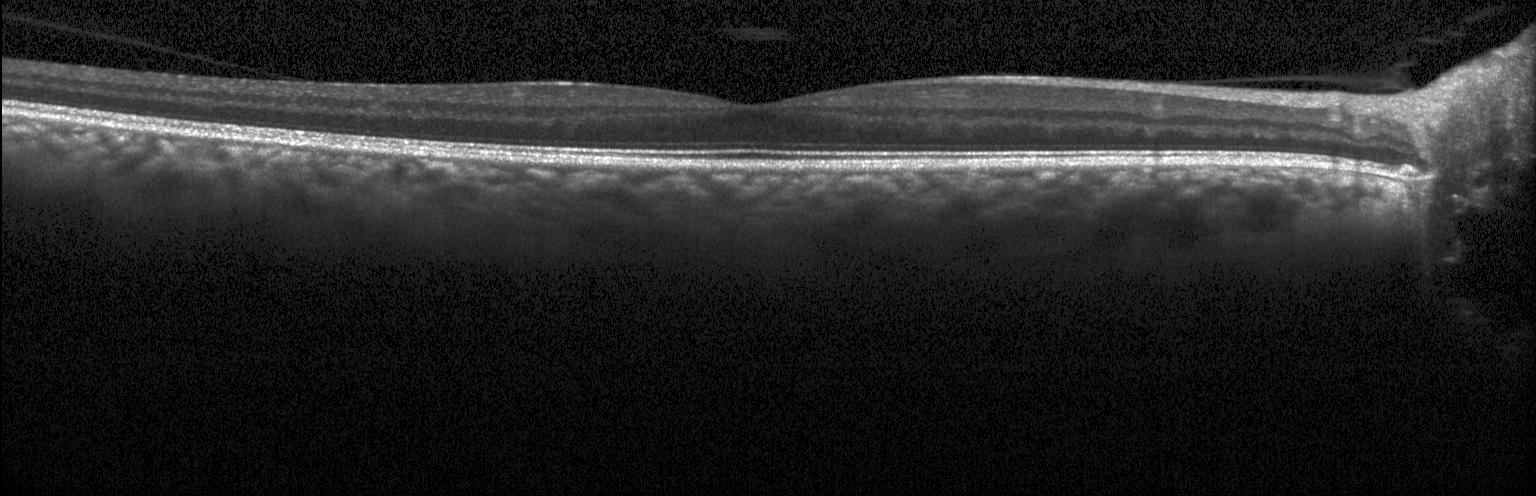

Impression: no CNV, no DME, and no drusen.